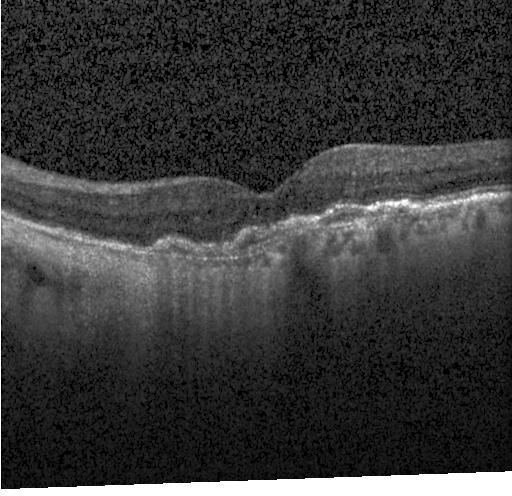 A choroidal neovascular membrane.